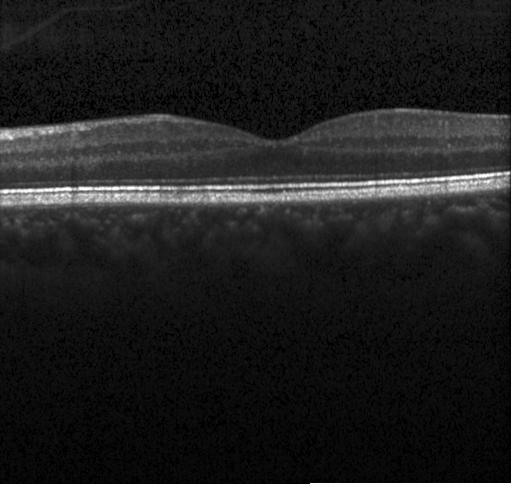 Acquired on a Heidelberg Spectralis; OCT B-scan; SD-OCT.
Diagnosis: no CNV, DME, or drusen.